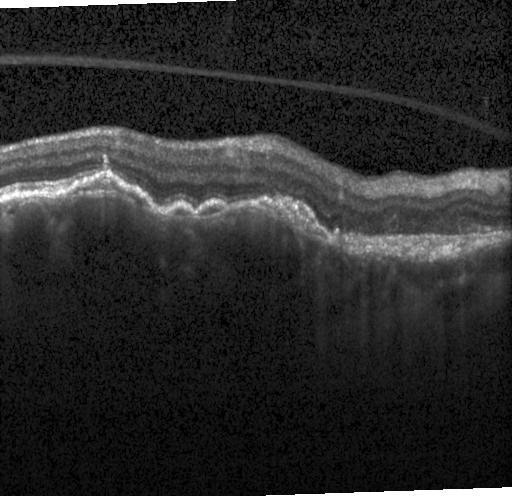
Assessment: a choroidal neovascular membrane.